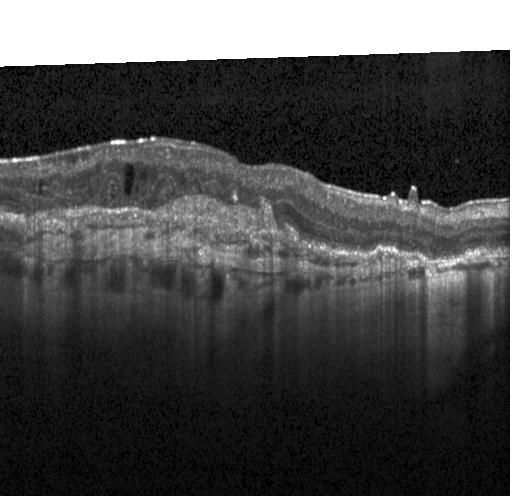 Macular scan. Spectral-domain OCT. Optical coherence tomography B-scan.
Impression: a choroidal neovascular membrane.